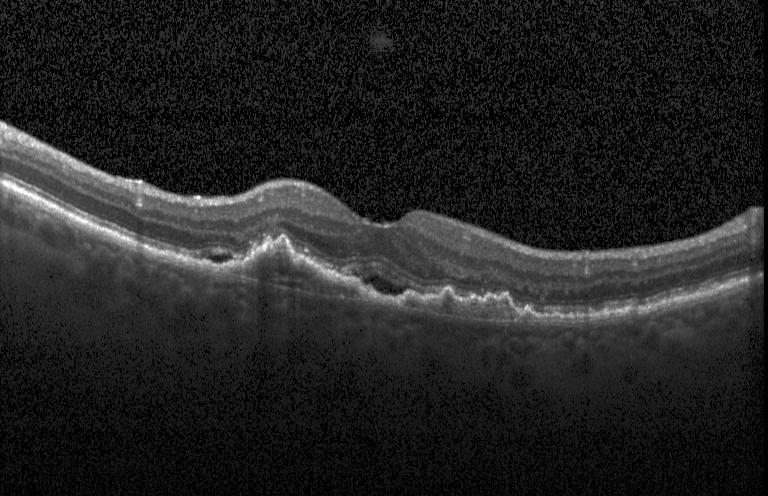
Optical coherence tomography scan, centered on the fovea — Dx: choroidal neovascularization.